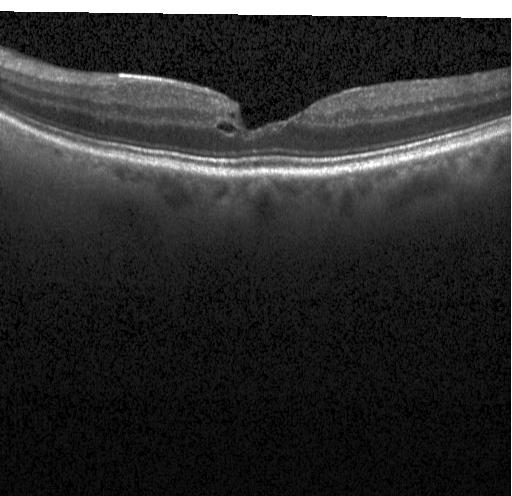 Spectral-domain OCT. Heidelberg Spectralis OCT system. OCT line scan. Finding: DME.